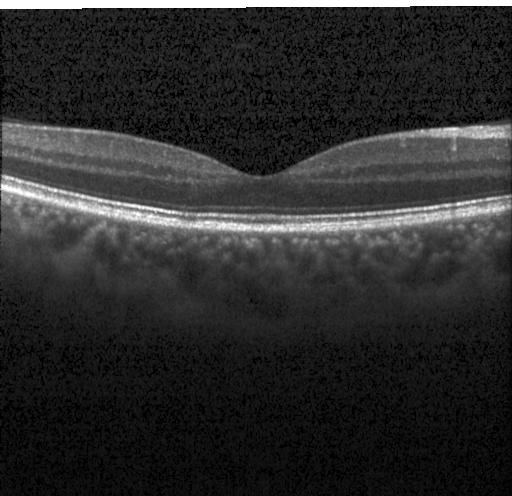
Optical coherence tomography scan
Diagnosis: no CNV, DME, or drusen.